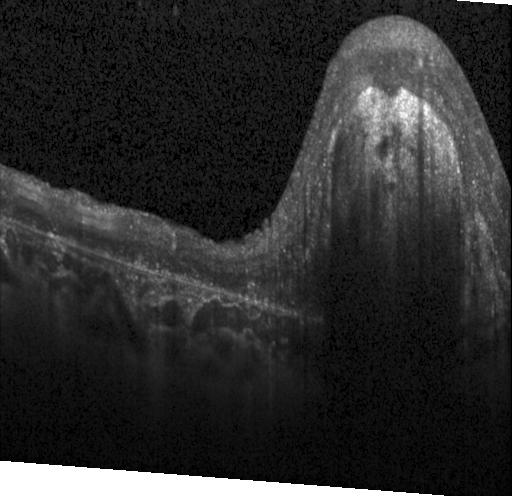
Heidelberg Spectralis OCT system, spectral-domain optical coherence tomography, retinal OCT cross-section, through the macula
Dx: choroidal neovascularization (CNV).